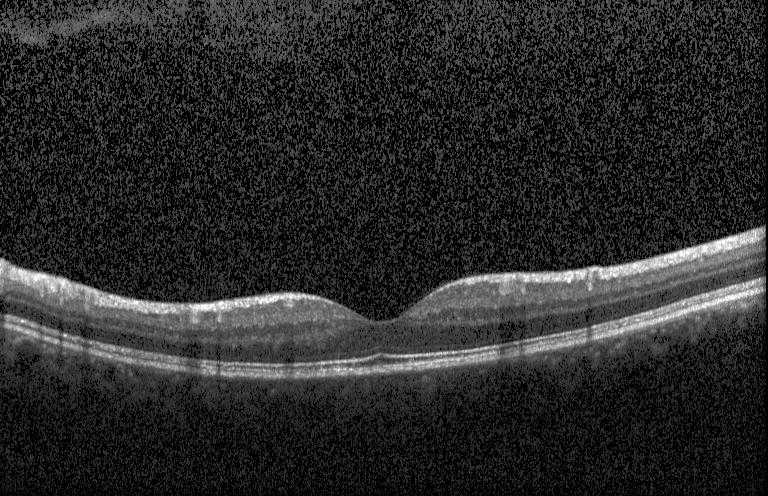

Finding: neither CNV, DME, nor drusen.